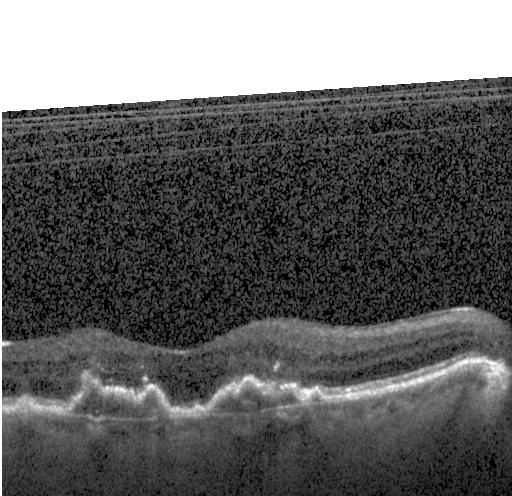 Macular OCT demonstrating a choroidal neovascular membrane.